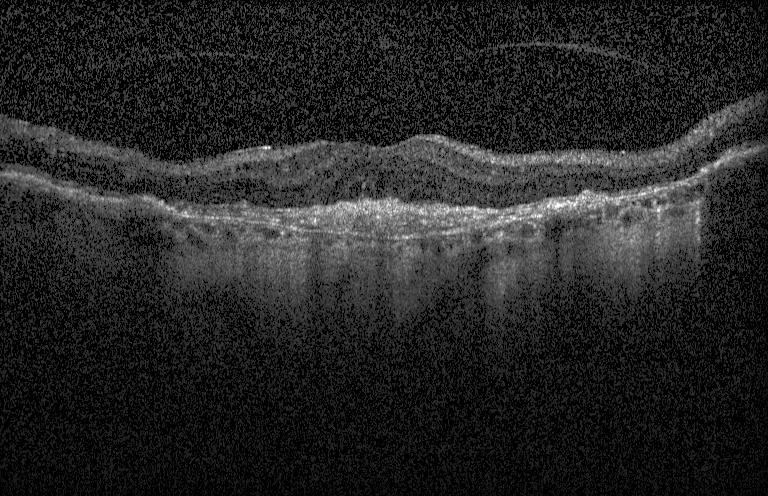 Retinal OCT cross-section showing a choroidal neovascular membrane.